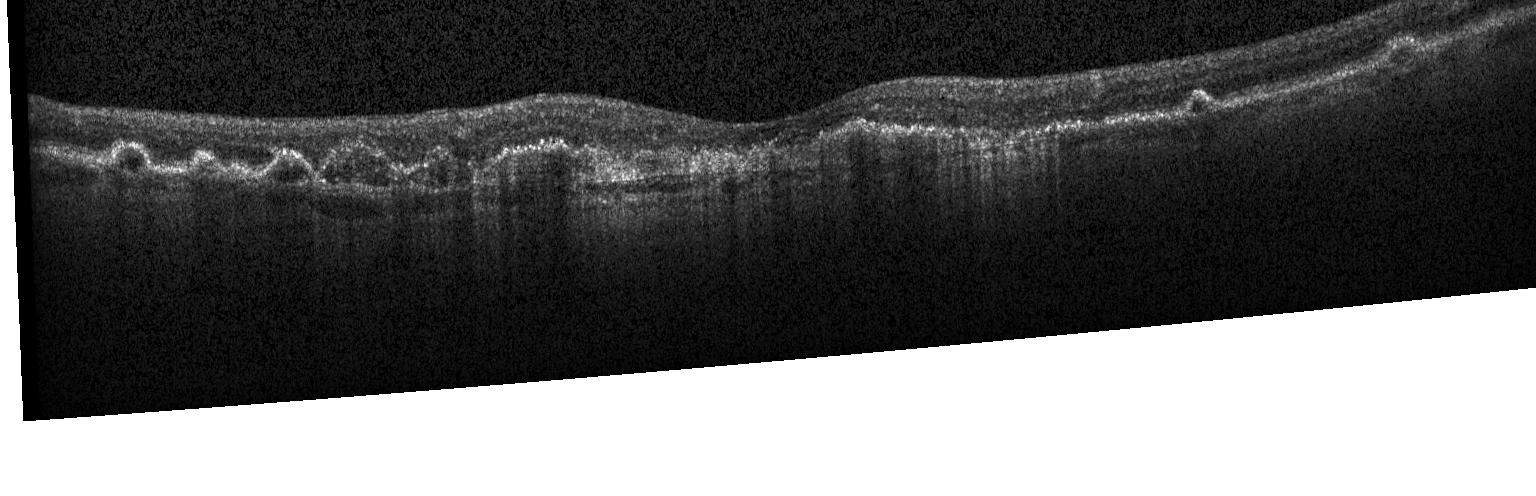

Retinal OCT B-scan, centered on the fovea, spectral-domain OCT.
Impression: a choroidal neovascular membrane.